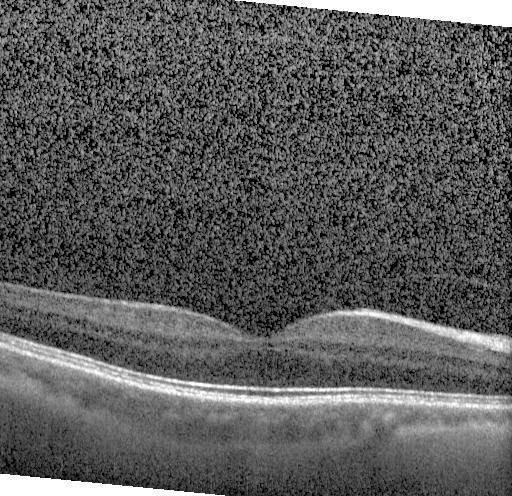 SD-OCT, optical coherence tomography scan, fovea-centered
Diagnosis: neither CNV, DME, nor drusen.